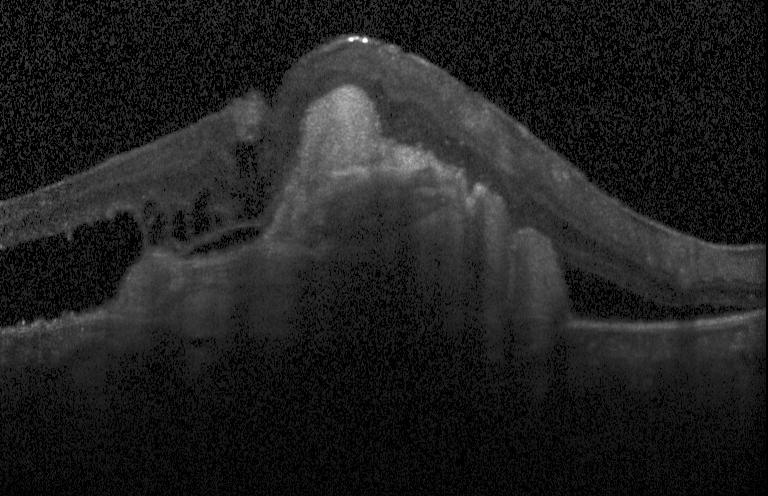

Optical coherence tomography B-scan — Impression: CNV.